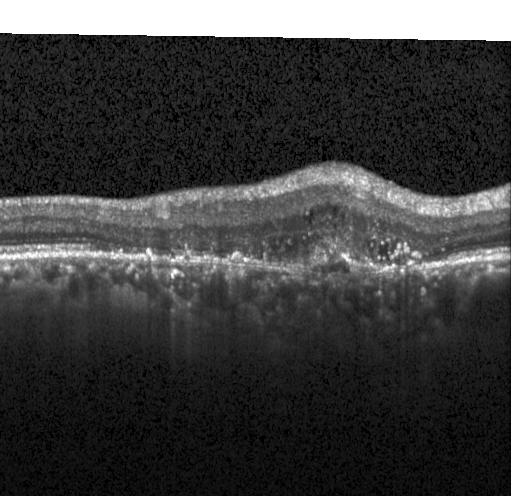 Spectral-domain OCT B-scan: a choroidal neovascular membrane.